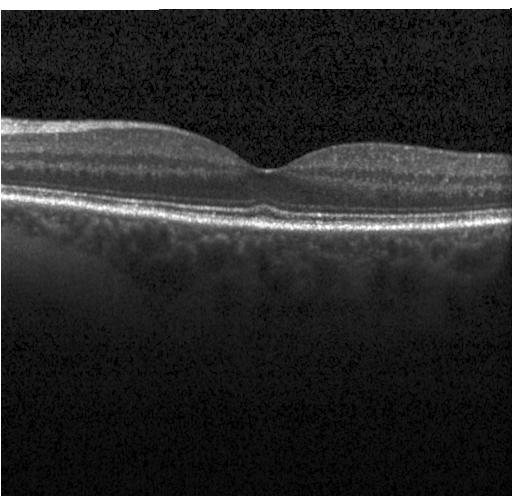
OCT finding: no choroidal neovascularization, no diabetic macular edema, and no drusen.